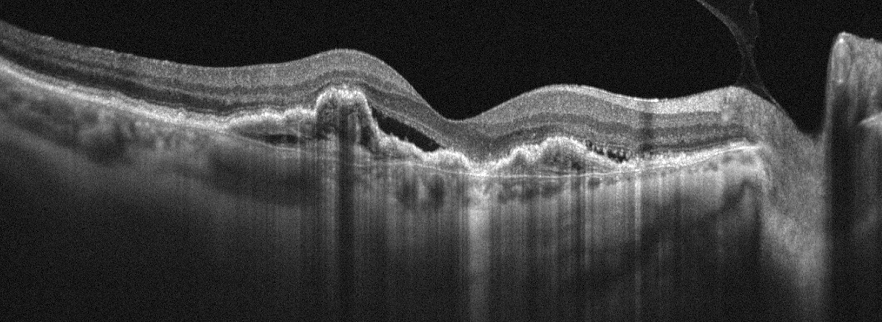 Optical coherence tomography B-scan.
The scan shows age-related macular degeneration (AMD).